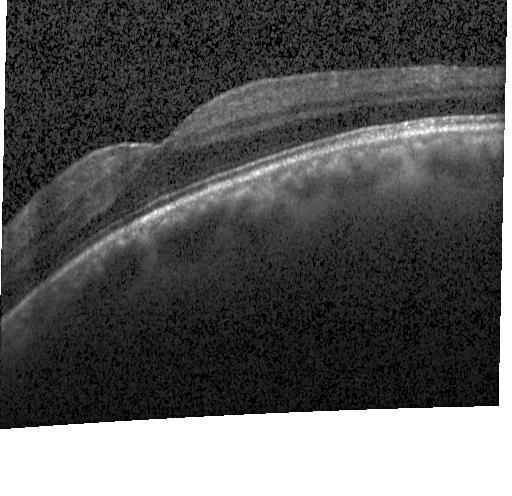
OCT line scan
Dx: neither CNV, DME, nor drusen.